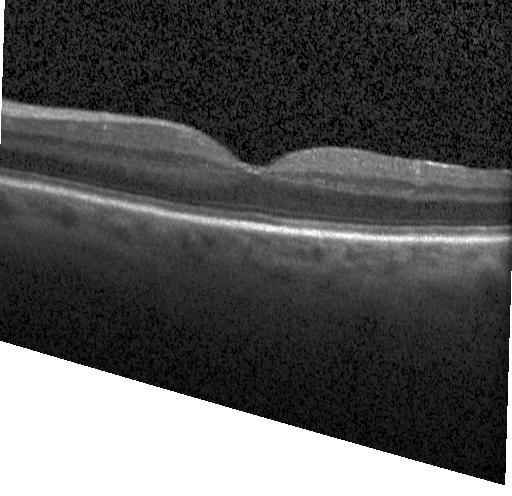
Retinal OCT B-scan — Assessment: no CNV, no DME, and no drusen.